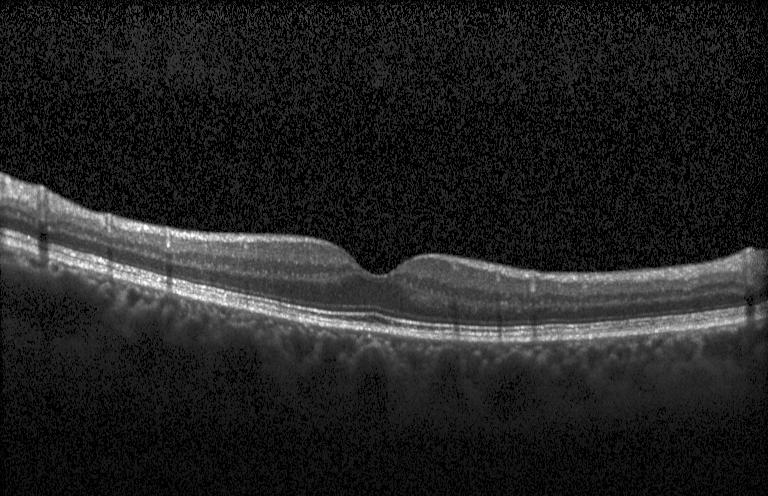

OCT line scan — Dx: neither choroidal neovascularization, diabetic macular edema, nor drusen.